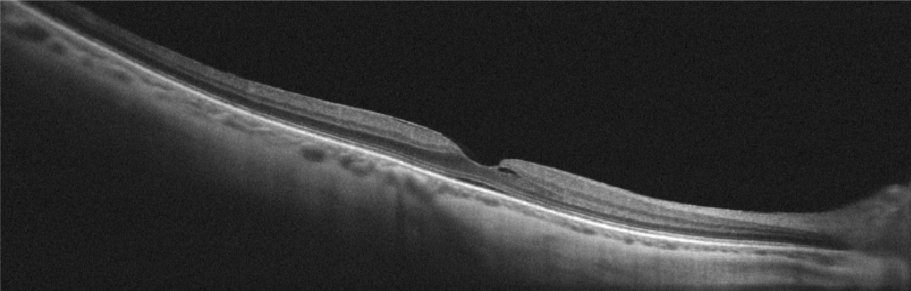
Macular scan · acquired on an Optovue Avanti RTVue XR · optical coherence tomography B-scan
Vitreomacular interface disease.